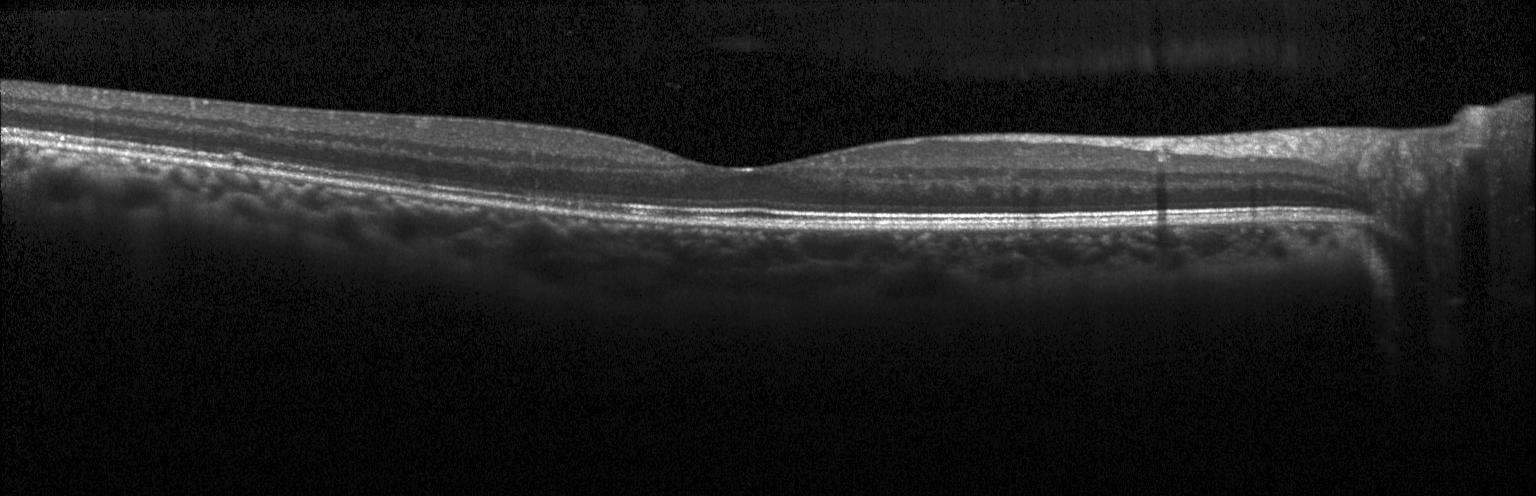
OCT scan showing no CNV, DME, or drusen.